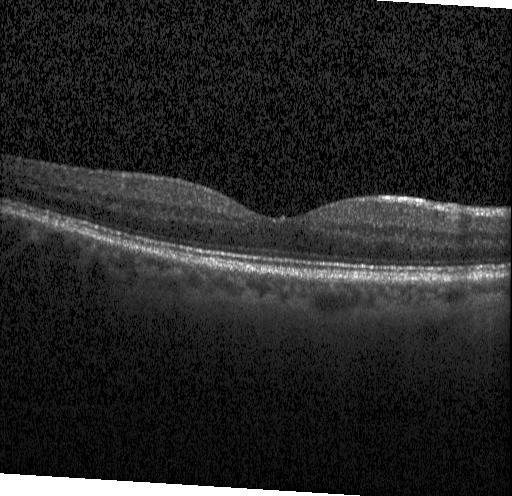
Retinal OCT B-scan — Diagnosis: neither choroidal neovascularization, diabetic macular edema, nor drusen.